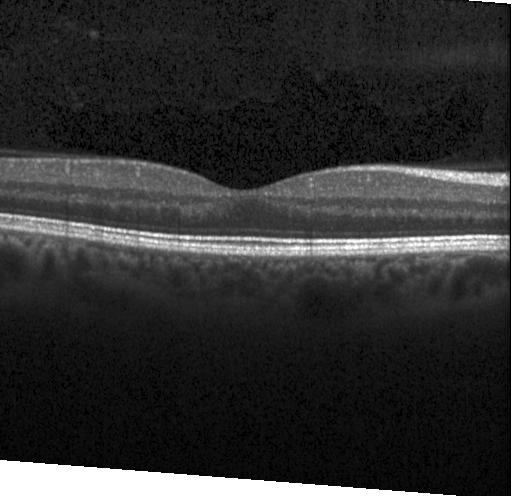
Retinal OCT B-scan
Diagnosis: neither choroidal neovascularization, diabetic macular edema, nor drusen.